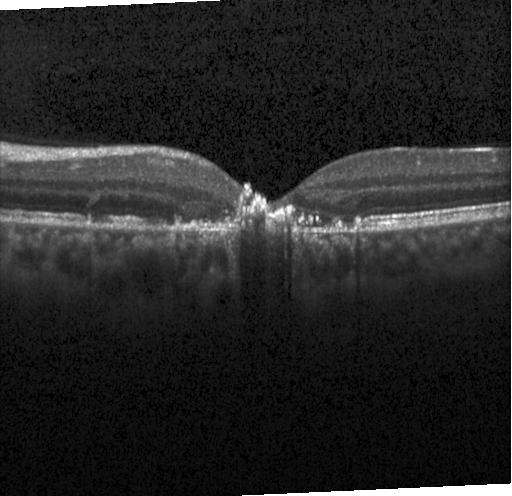 Heidelberg Spectralis OCT system; spectral-domain optical coherence tomography; retinal OCT B-scan. Finding: choroidal neovascularization (CNV).